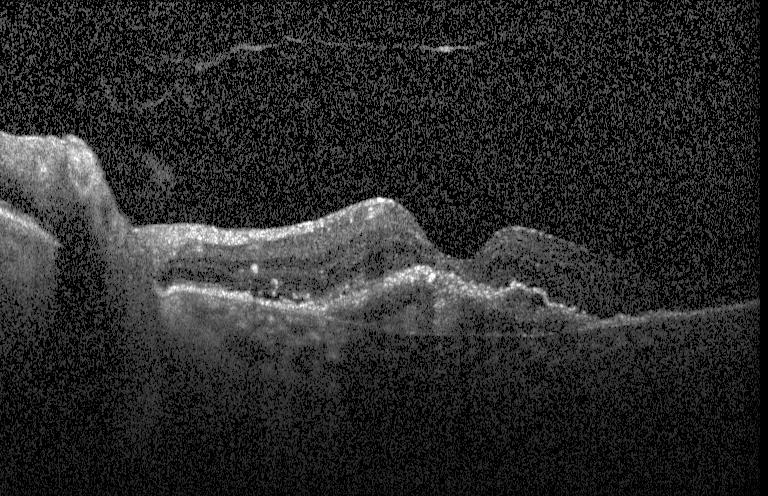
Instrument: Heidelberg Spectralis · centered on the fovea · optical coherence tomography B-scan.
Impression: CNV.